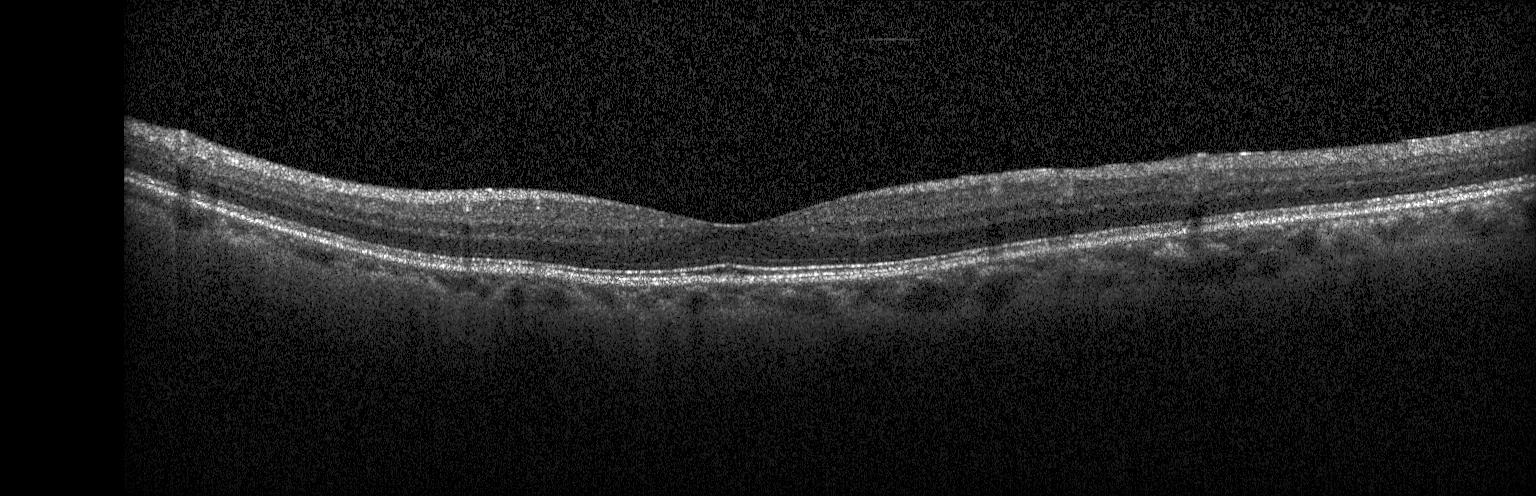

OCT B-scan — Diagnosis: no evidence of choroidal neovascularization, diabetic macular edema, or drusen.